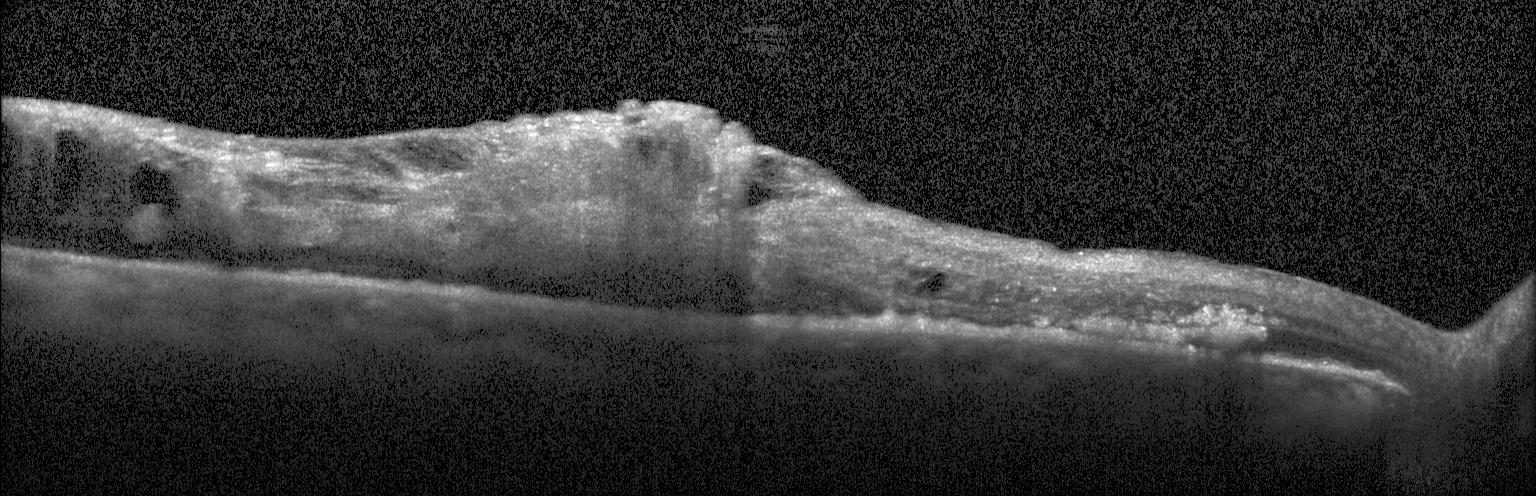 OCT B-scan. Assessment: choroidal neovascularization.